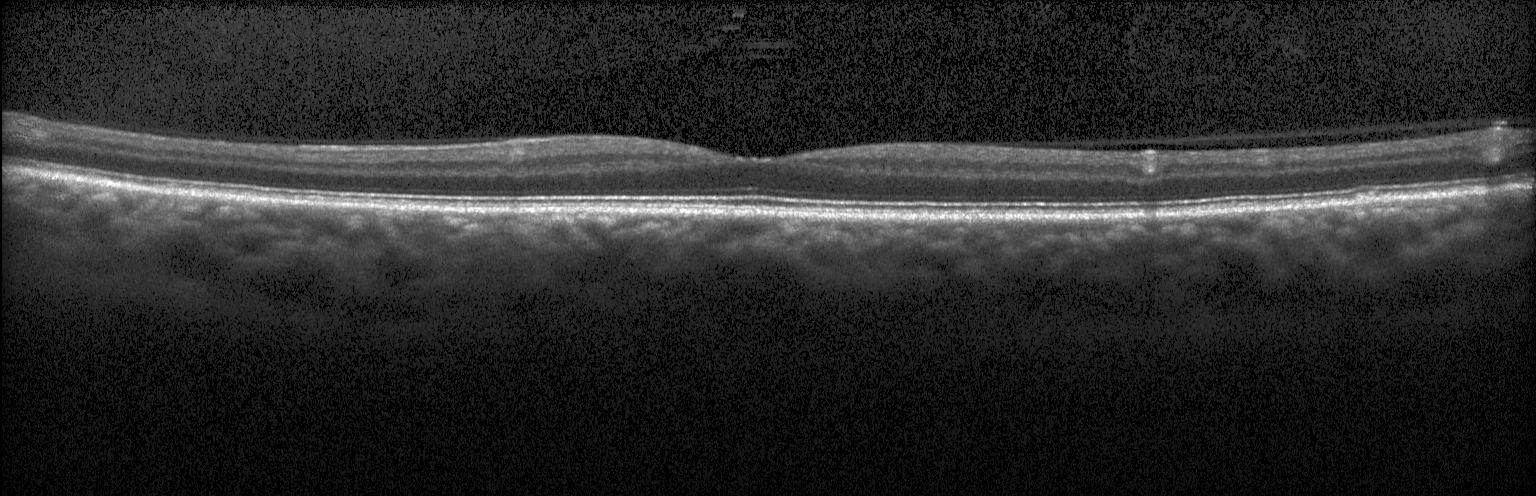 Spectral-domain optical coherence tomography, OCT B-scan.
No choroidal neovascularization, diabetic macular edema, or drusen.